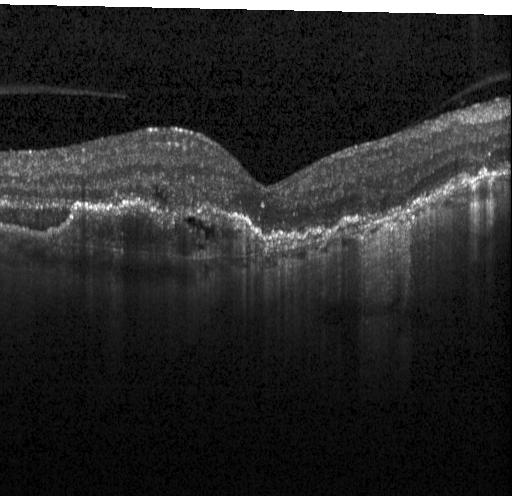
Impression: choroidal neovascularization (CNV).